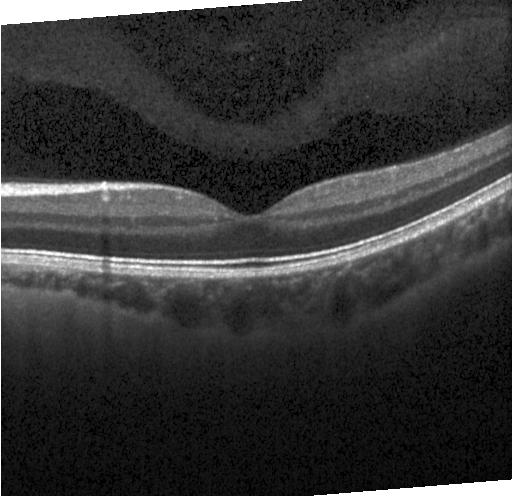 Acquired on a Heidelberg Spectralis, SD-OCT, optical coherence tomography scan, macular scan. Finding: no choroidal neovascularization, no diabetic macular edema, and no drusen.